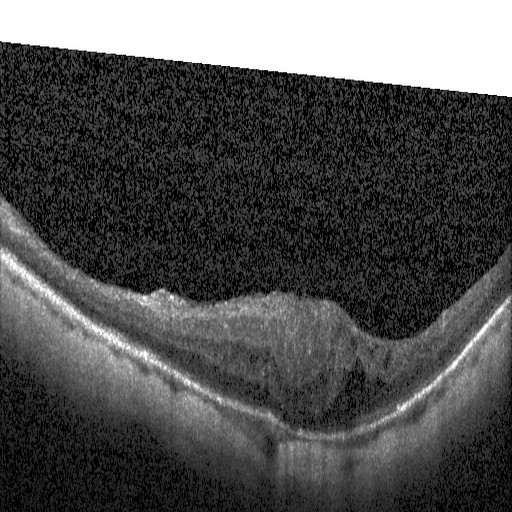
OCT scan showing diabetic macular edema.